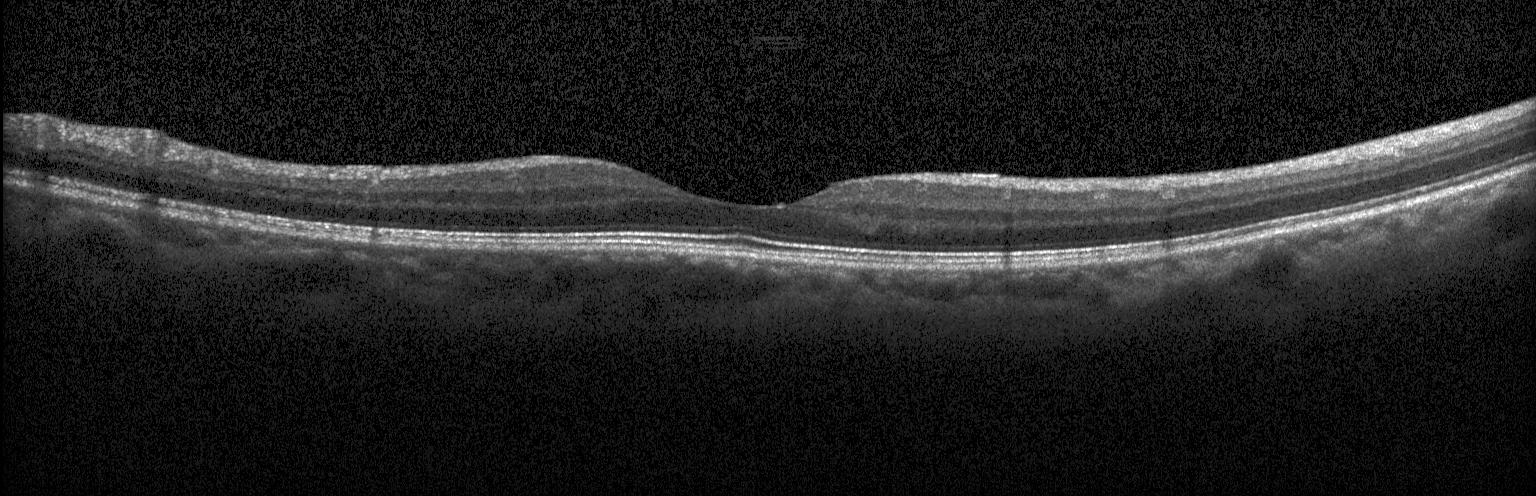 Retinal OCT cross-section, spectral-domain optical coherence tomography, through the macula, instrument: Heidelberg Spectralis
Impression: neither choroidal neovascularization, diabetic macular edema, nor drusen.